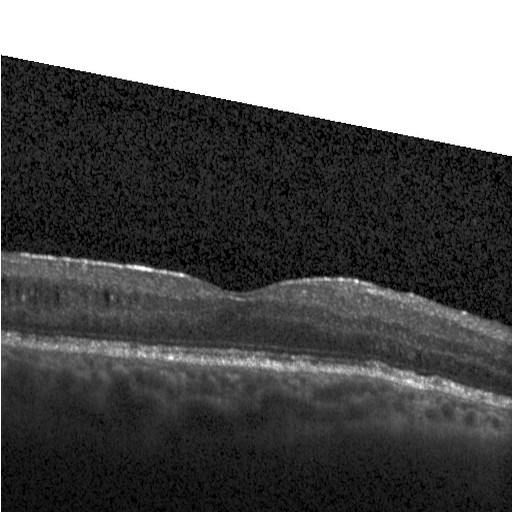

Optical coherence tomography scan
Finding: diabetic macular edema (DME).